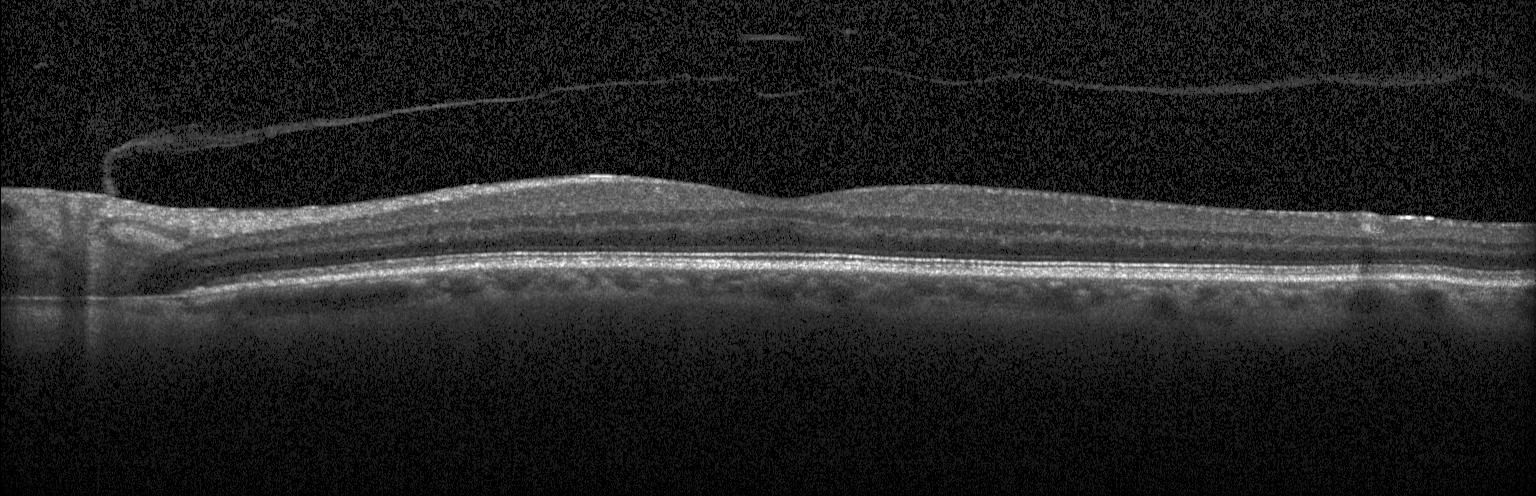

Diagnosis: no choroidal neovascularization, no diabetic macular edema, and no drusen.